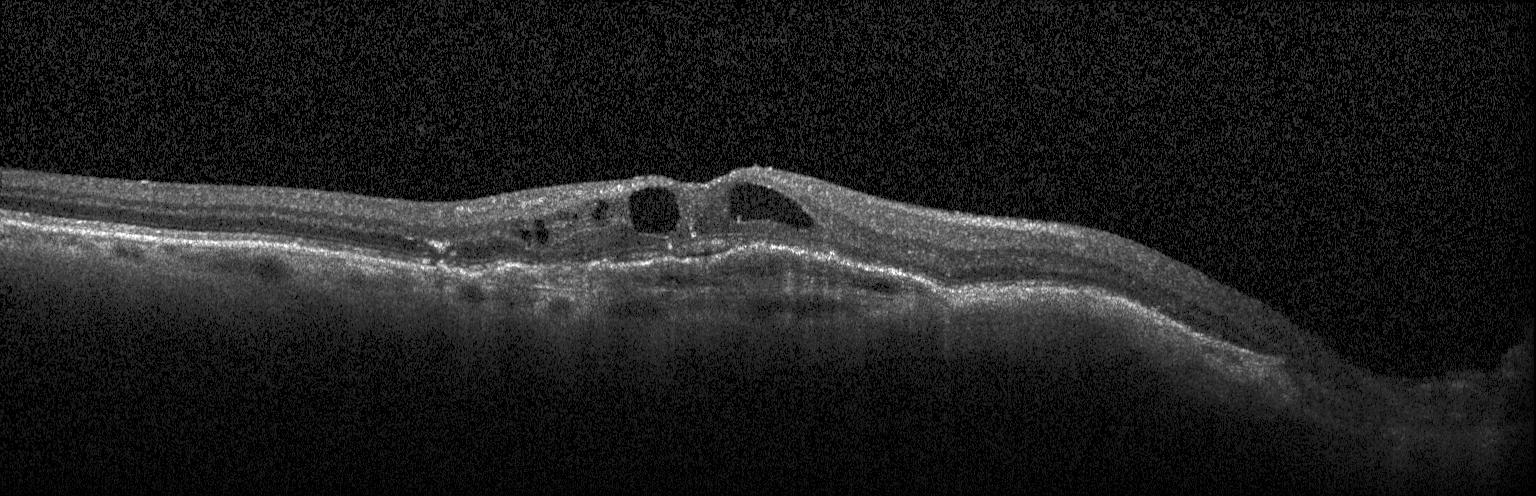 SD-OCT · OCT B-scan. A choroidal neovascular membrane.